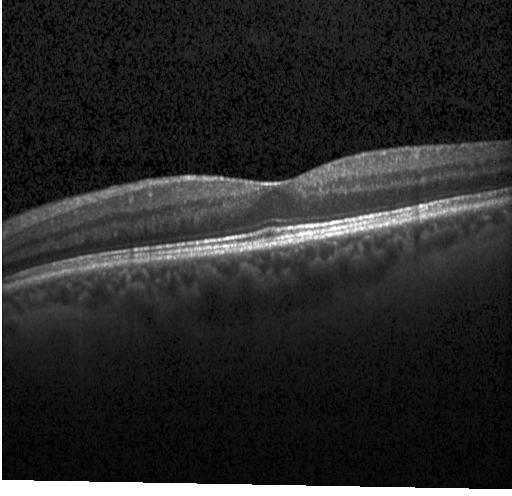
Macular OCT demonstrating no choroidal neovascularization, no diabetic macular edema, and no drusen.